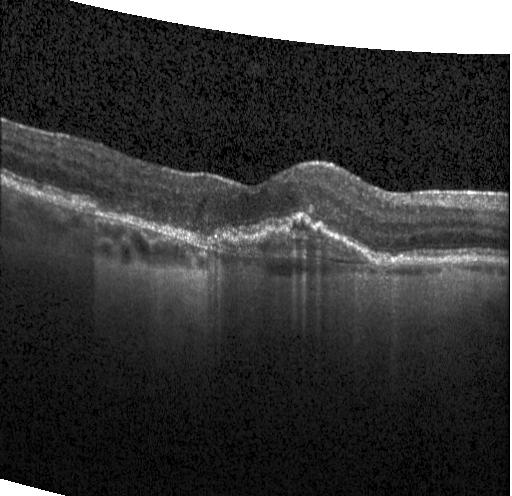

OCT finding: choroidal neovascularization (CNV).